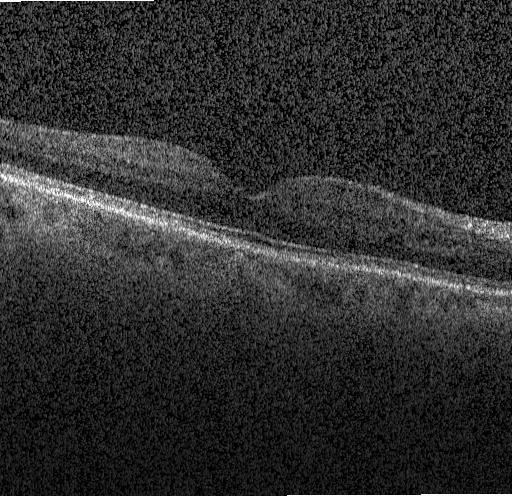
Impression: neither choroidal neovascularization, diabetic macular edema, nor drusen.